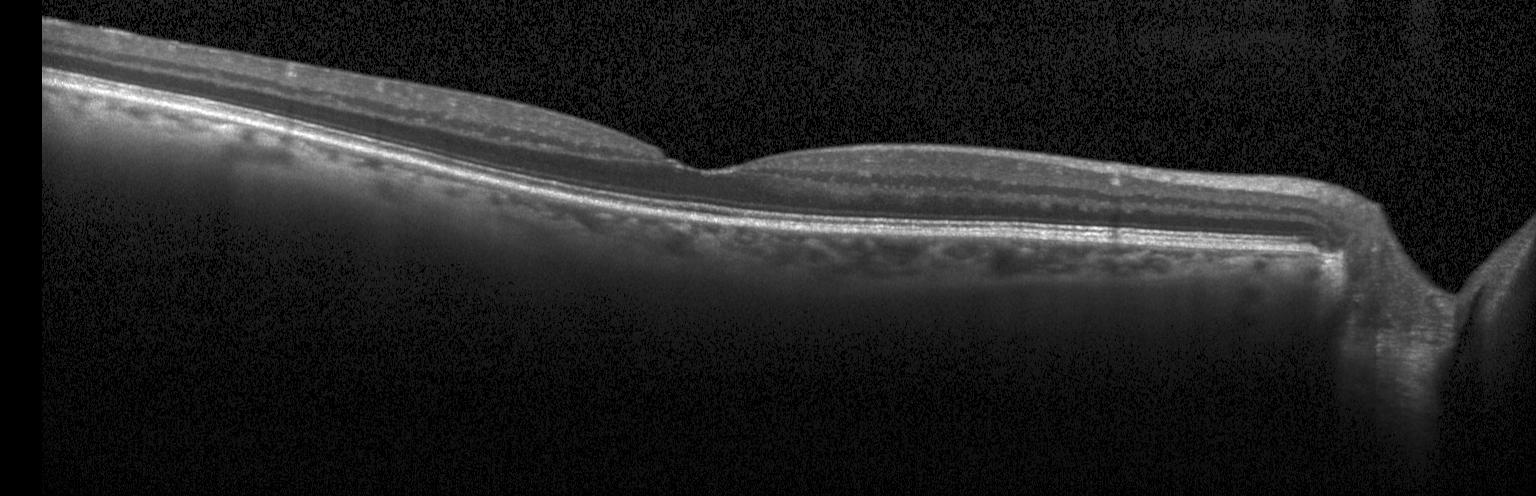

OCT B-scan showing no evidence of choroidal neovascularization, diabetic macular edema, or drusen.